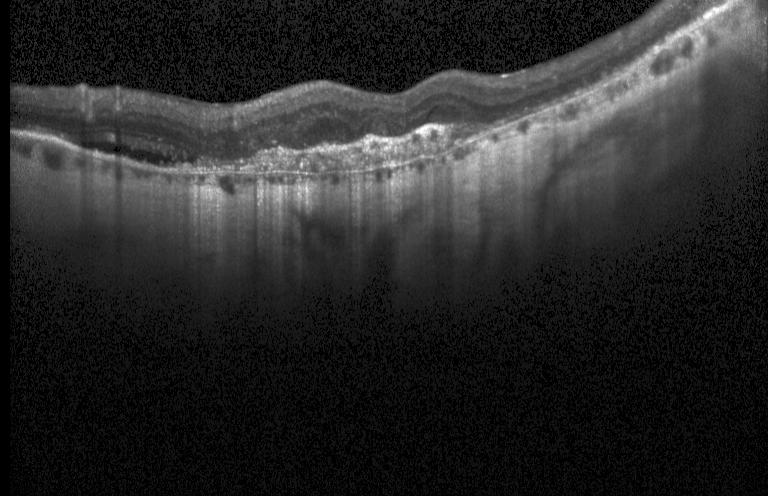
Optical coherence tomography scan; macular scan; spectral-domain optical coherence tomography — OCT finding: choroidal neovascularization (CNV).